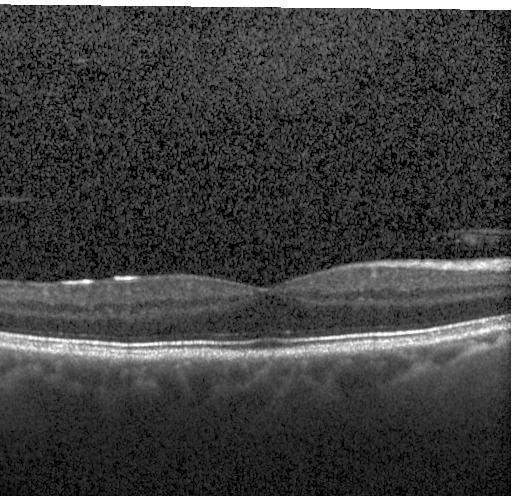 Fovea-centered, retinal OCT B-scan, Heidelberg Spectralis, spectral-domain optical coherence tomography.
Impression: neither choroidal neovascularization, diabetic macular edema, nor drusen.